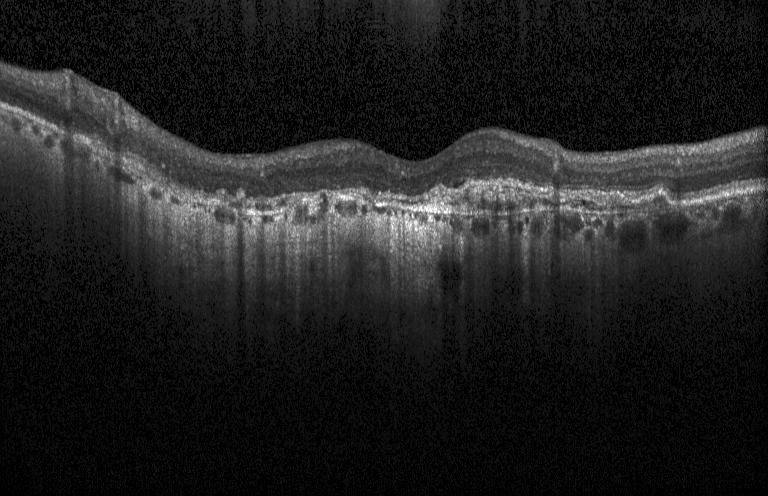 Centered on the fovea, SD-OCT, retinal OCT cross-section. Diagnosis: a choroidal neovascular membrane.